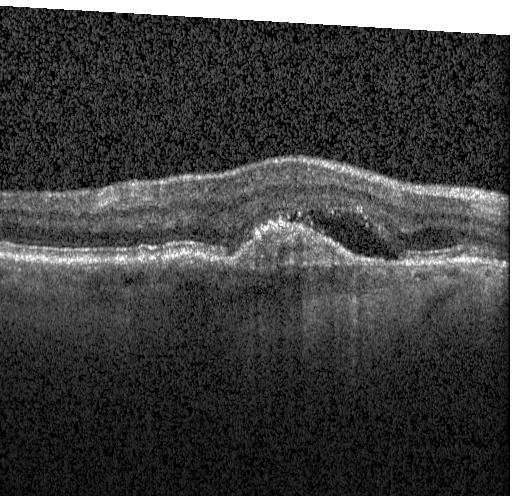 Horizontal scan through the fovea. Retinal OCT B-scan — Impression: a choroidal neovascular membrane.